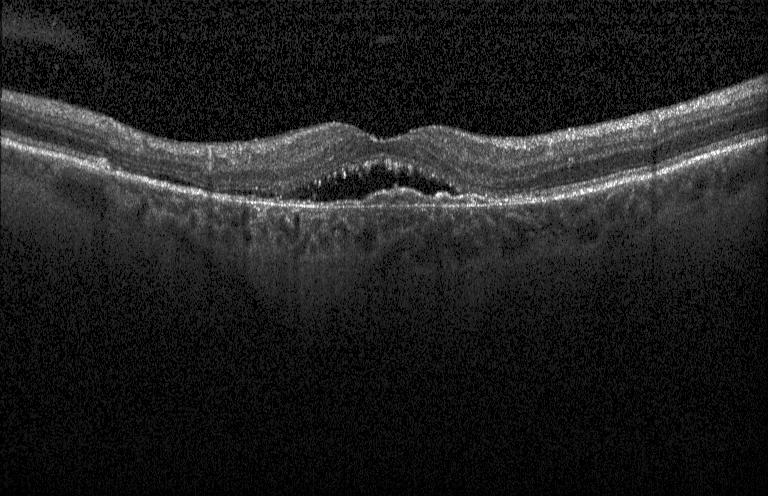
Spectral-domain optical coherence tomography; optical coherence tomography B-scan
The scan shows a choroidal neovascular membrane.